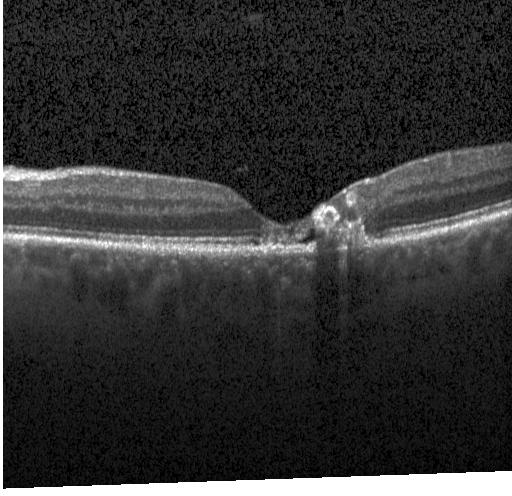

OCT B-scan showing a choroidal neovascular membrane.